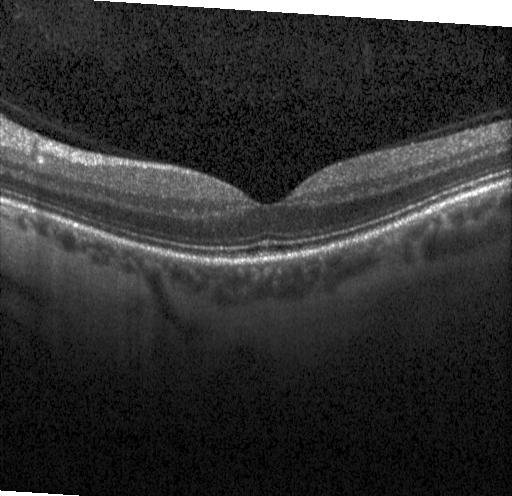 Optical coherence tomography B-scan — Macular OCT: neither CNV, DME, nor drusen.